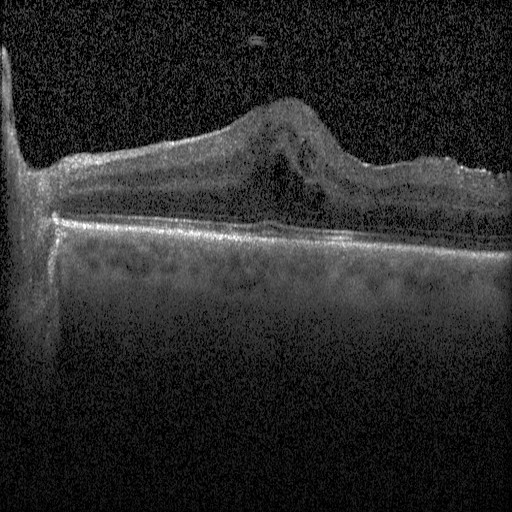
Optical coherence tomography B-scan
Macular OCT: diabetic macular edema.